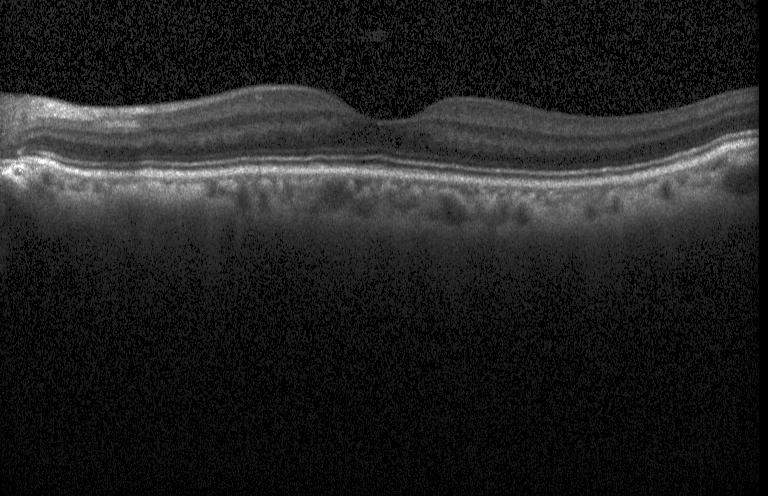

Impression: no evidence of choroidal neovascularization, diabetic macular edema, or drusen.